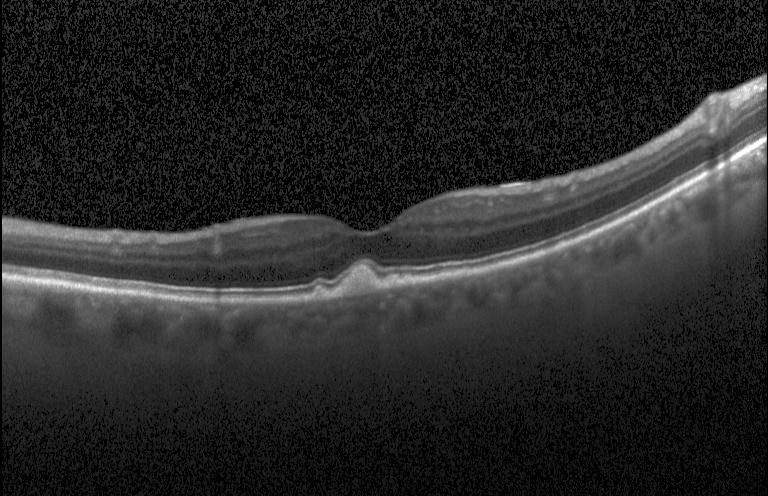

Diagnosis: drusen.